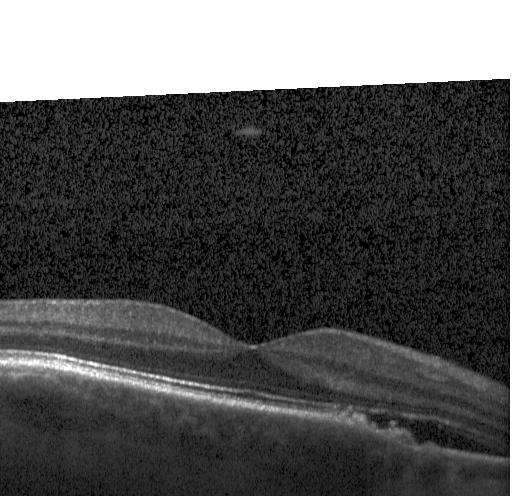
Diagnosis: choroidal neovascularization.